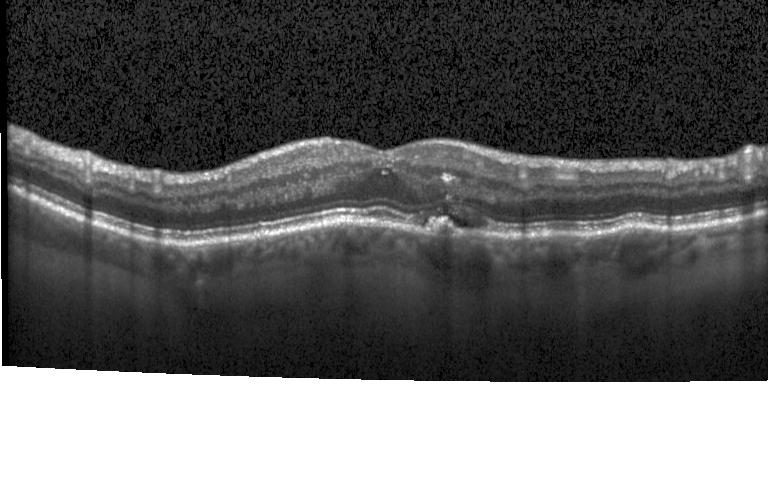

Finding: a choroidal neovascular membrane.